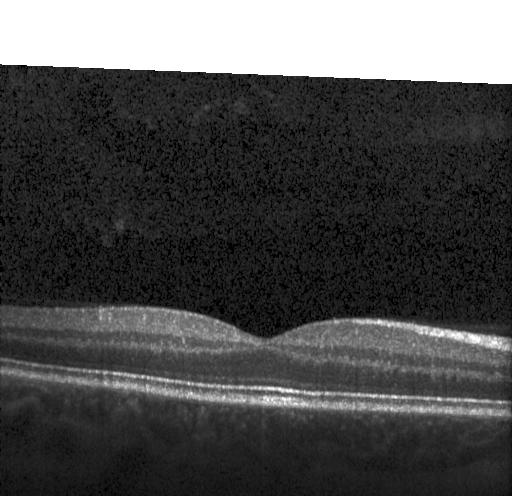
Impression: no choroidal neovascularization, diabetic macular edema, or drusen.